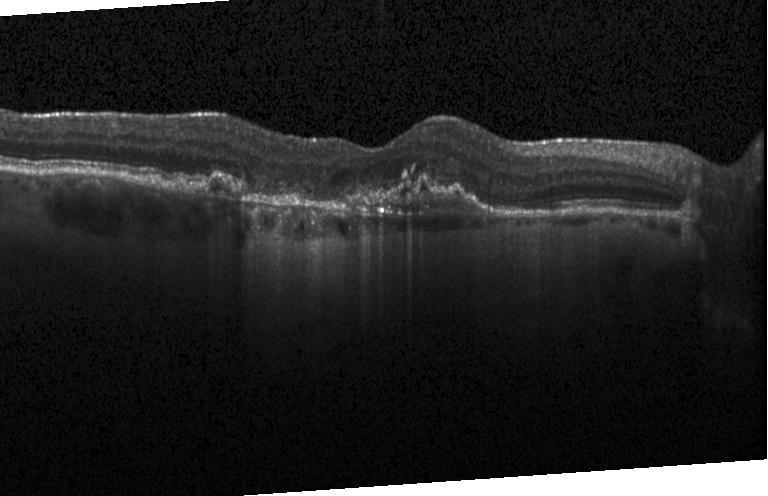 OCT finding: a choroidal neovascular membrane.